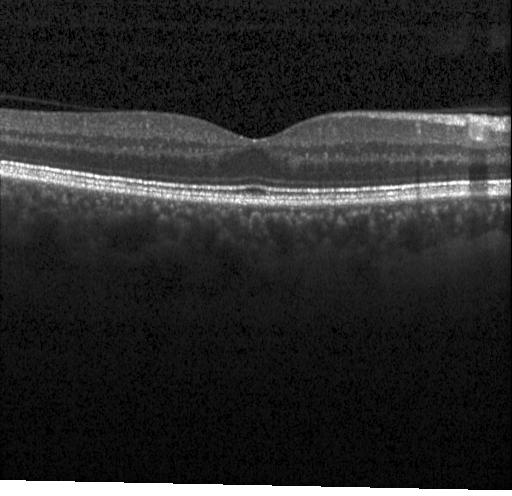 Assessment: no evidence of choroidal neovascularization, diabetic macular edema, or drusen.